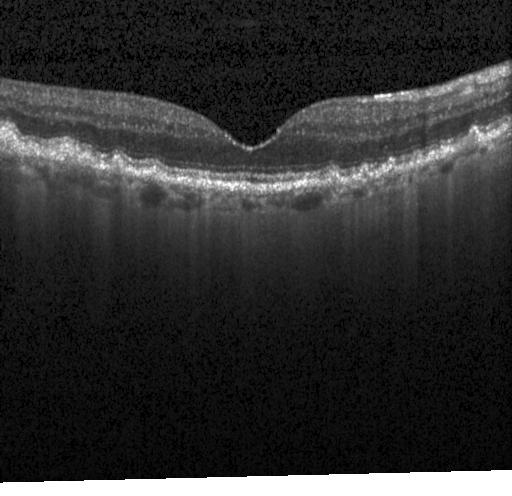 Retinal OCT B-scan — The scan shows drusen.